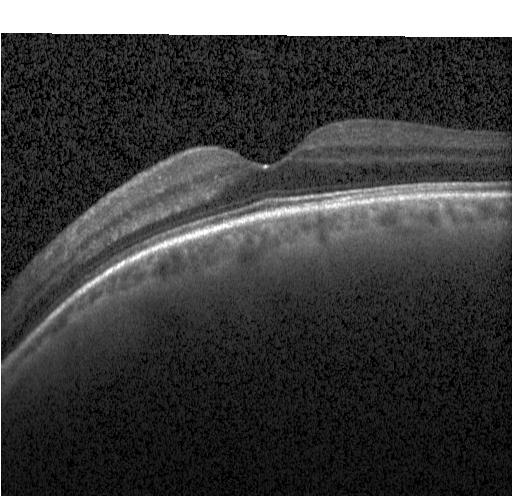
OCT scan showing no choroidal neovascularization, diabetic macular edema, or drusen.